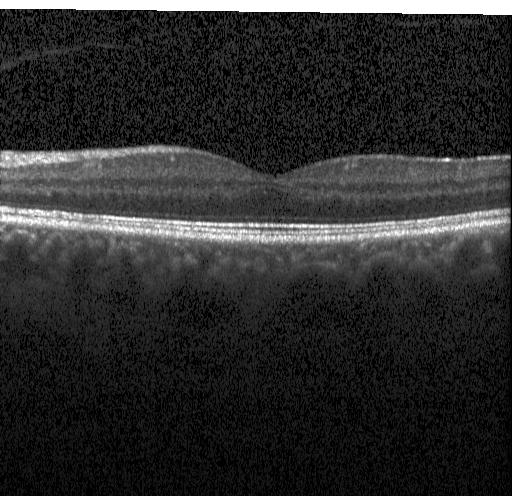
Diagnosis: no choroidal neovascularization, diabetic macular edema, or drusen.